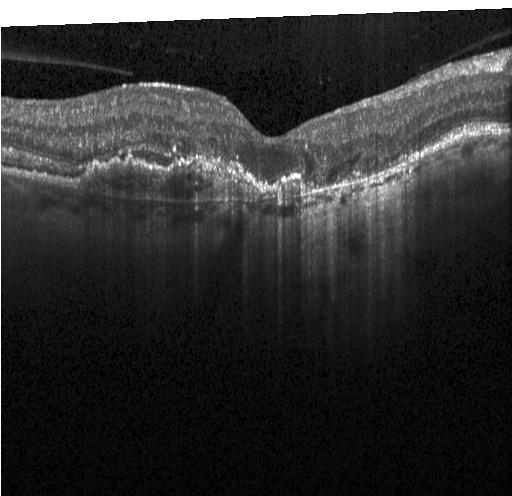 Retinal OCT B-scan
The scan shows choroidal neovascularization.